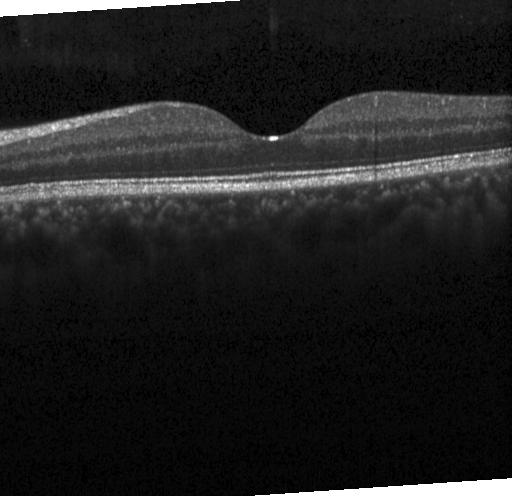 OCT line scan
Finding: no choroidal neovascularization, diabetic macular edema, or drusen.